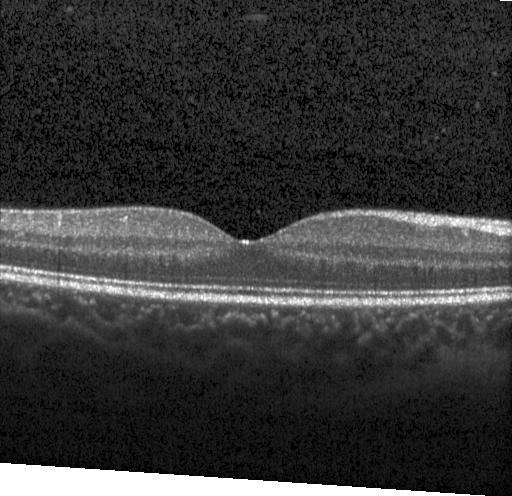

Optical coherence tomography B-scan.
No choroidal neovascularization, diabetic macular edema, or drusen.